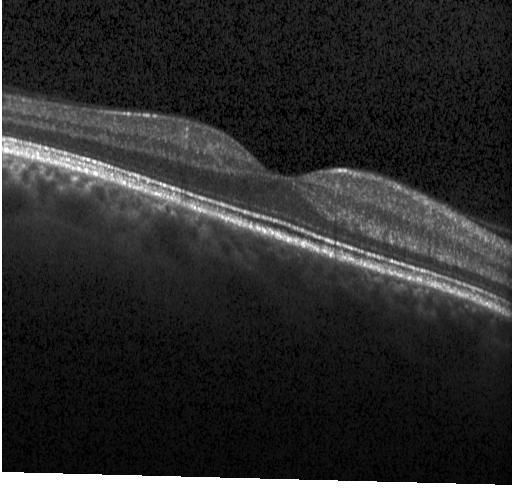
Assessment: neither CNV, DME, nor drusen.